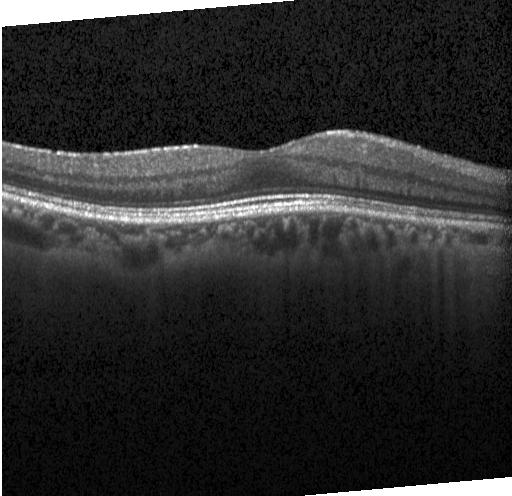 Macular OCT: no choroidal neovascularization, diabetic macular edema, or drusen.